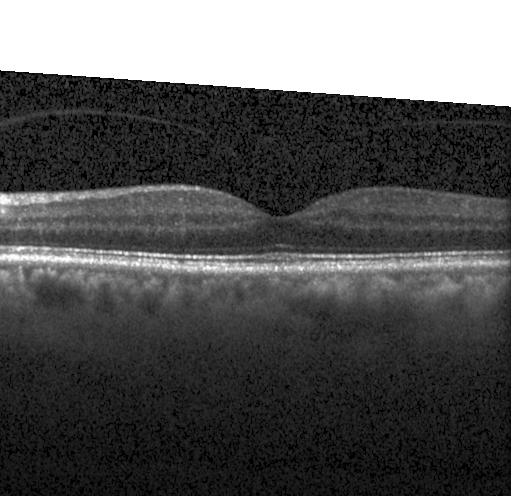

Acquired on a Heidelberg Spectralis · OCT line scan · spectral-domain OCT
Finding: no choroidal neovascularization, diabetic macular edema, or drusen.